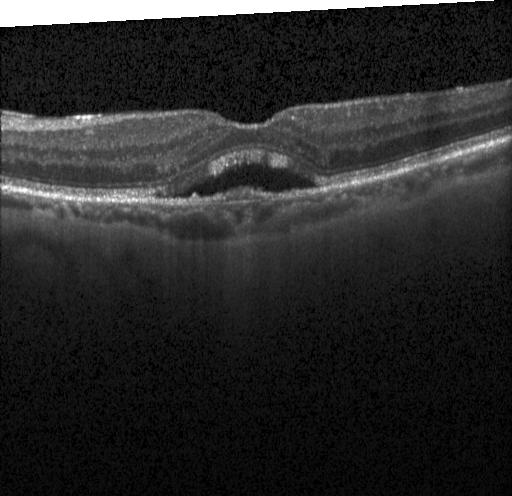
Spectral-domain OCT B-scan: a choroidal neovascular membrane.